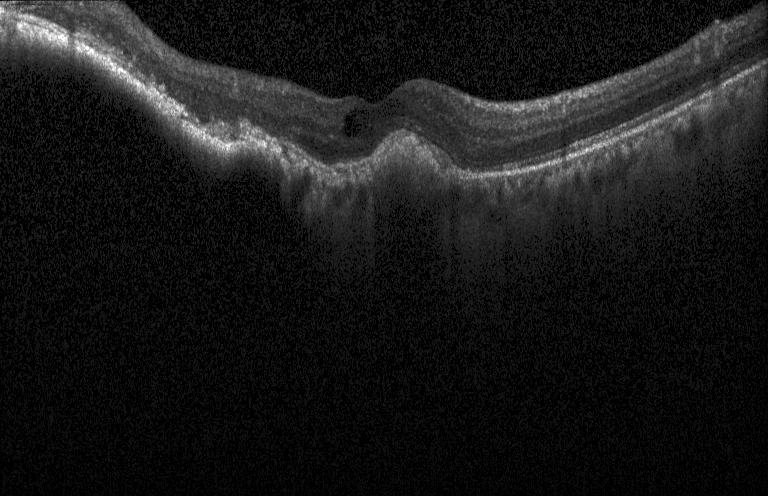 Retinal OCT cross-section. Impression: choroidal neovascularization (CNV).